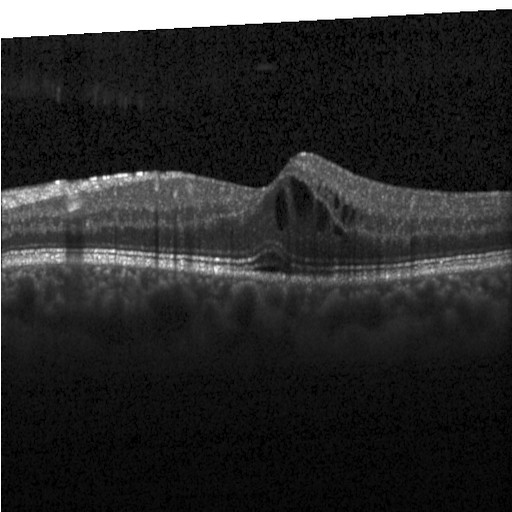 OCT scan showing diabetic macular edema.